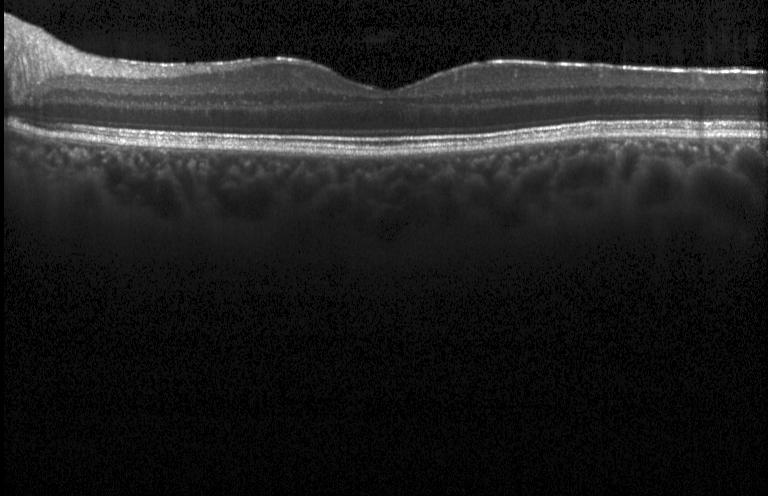
OCT line scan.
Diagnosis: no CNV, DME, or drusen.